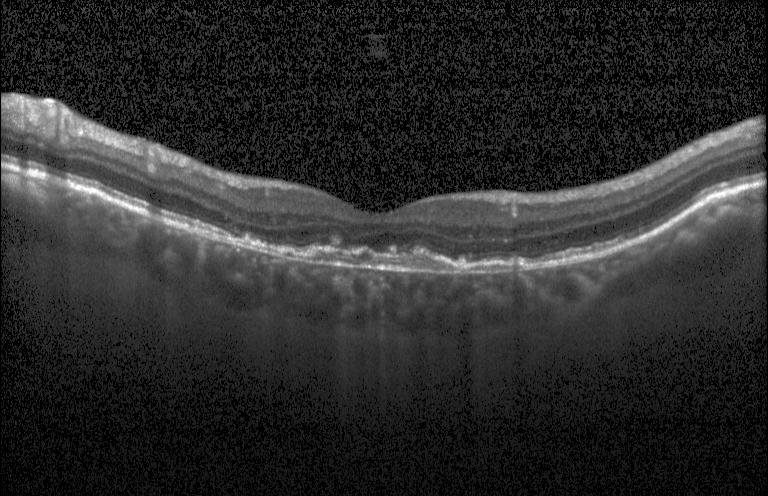 OCT B-scan — Impression: a choroidal neovascular membrane.